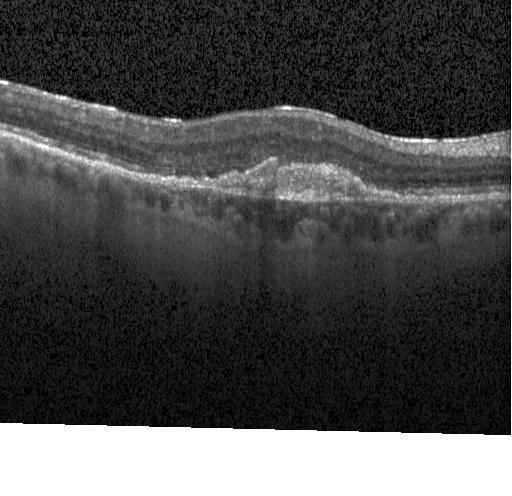
Horizontal scan through the fovea, optical coherence tomography scan — This B-scan demonstrates a choroidal neovascular membrane.